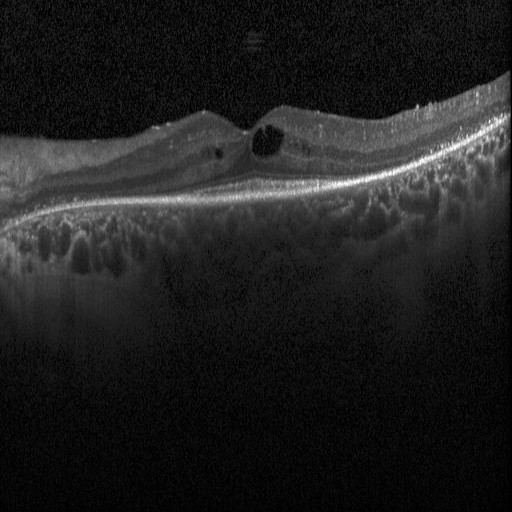 Macular OCT: DME.